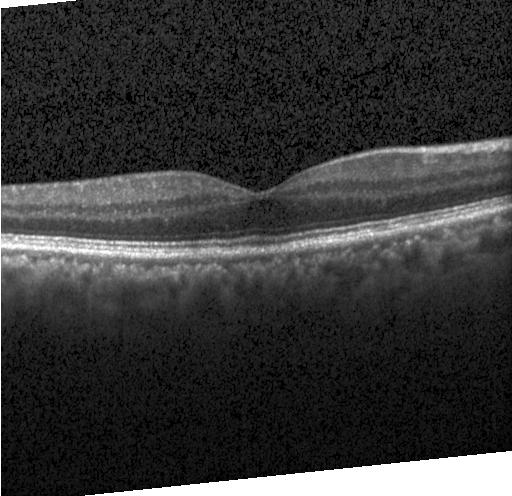

Finding: neither choroidal neovascularization, diabetic macular edema, nor drusen.